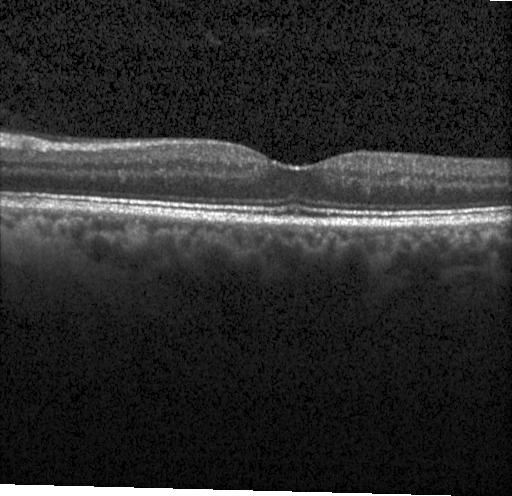

OCT B-scan, instrument: Heidelberg Spectralis, spectral-domain optical coherence tomography, centered on the fovea. OCT finding: no CNV, no DME, and no drusen.